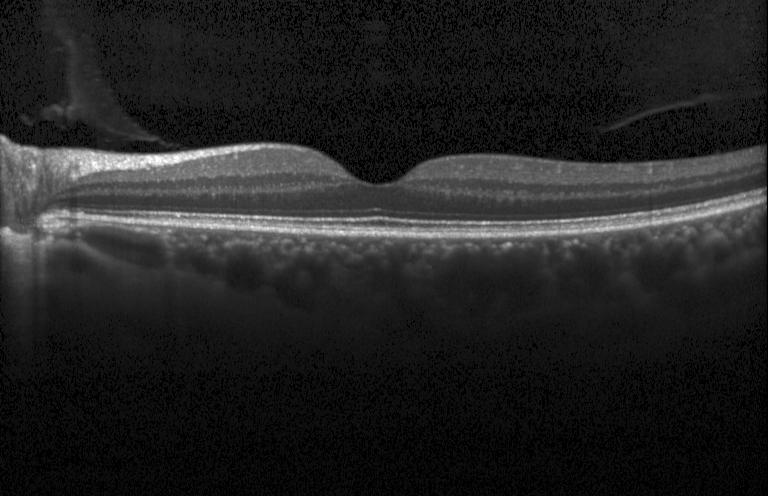

Heidelberg Spectralis OCT system; optical coherence tomography scan — OCT finding: neither choroidal neovascularization, diabetic macular edema, nor drusen.